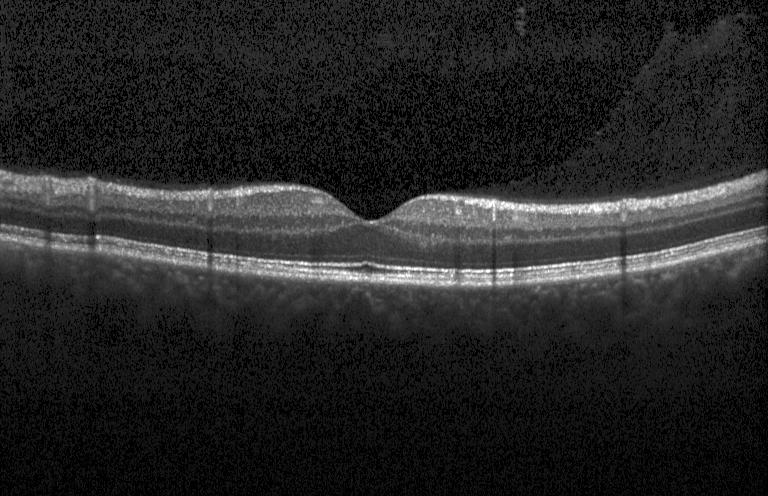 Diagnosis: no CNV, no DME, and no drusen.